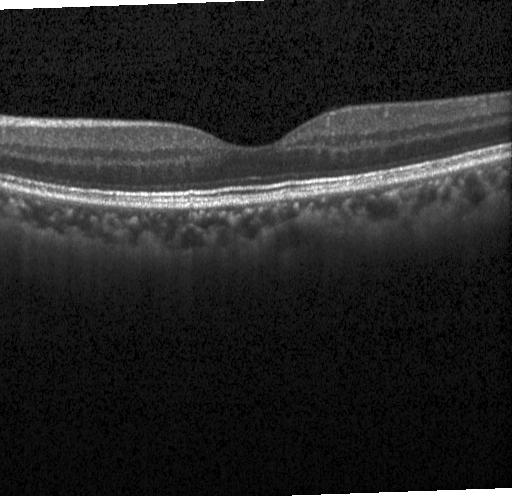

Impression: no evidence of CNV, DME, or drusen.